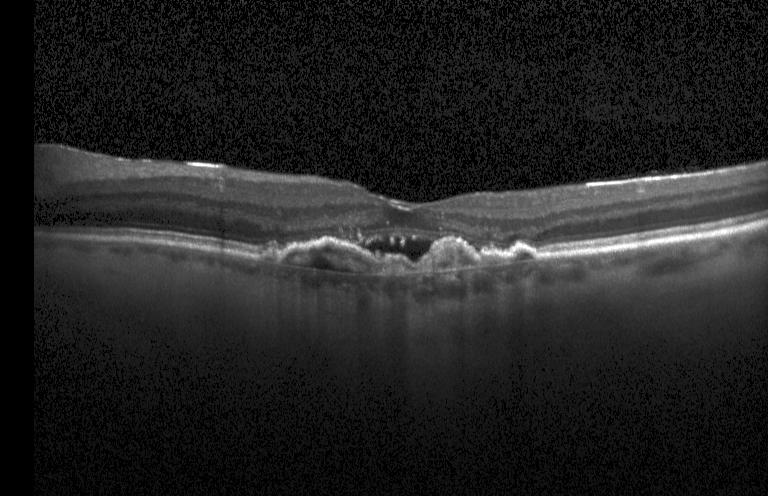
OCT B-scan showing CNV.